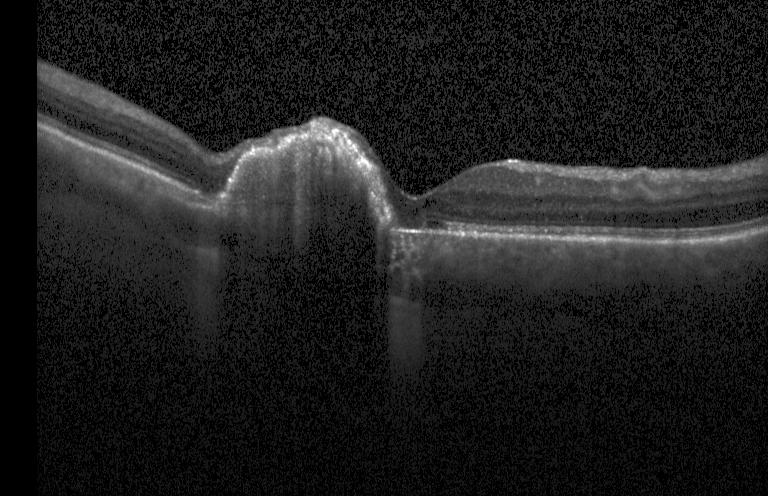

Through the macula · Heidelberg Spectralis · SD-OCT · optical coherence tomography scan.
Diagnosis: a choroidal neovascular membrane.